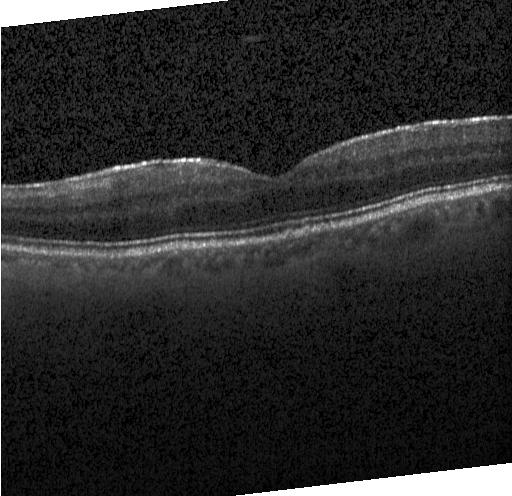 Spectral-domain optical coherence tomography; retinal OCT cross-section; through the macula — Macular OCT: no evidence of choroidal neovascularization, diabetic macular edema, or drusen.